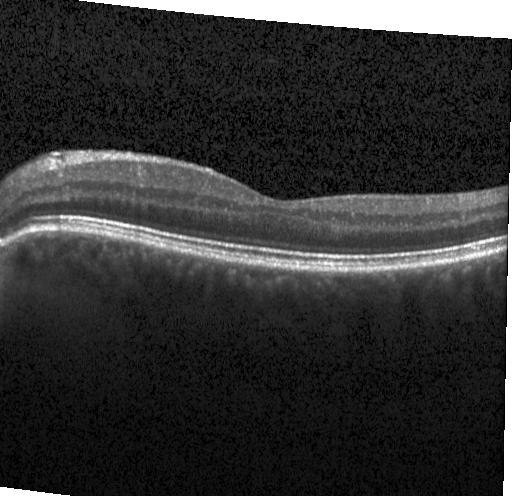
OCT line scan
No evidence of CNV, DME, or drusen.